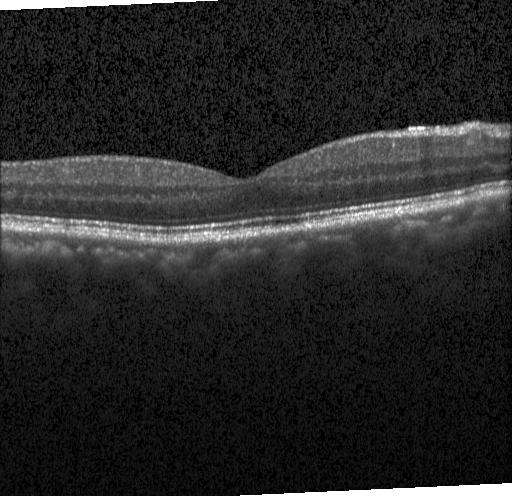 Finding: neither CNV, DME, nor drusen.